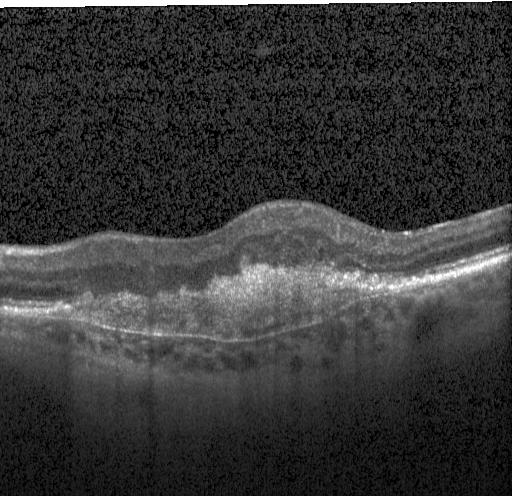

Acquired on a Heidelberg Spectralis; spectral-domain optical coherence tomography; optical coherence tomography B-scan
This B-scan demonstrates a choroidal neovascular membrane.